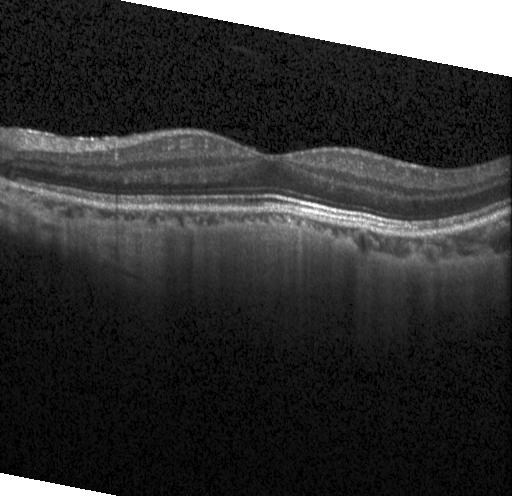
Retinal OCT cross-section; spectral-domain optical coherence tomography.
No choroidal neovascularization, diabetic macular edema, or drusen.